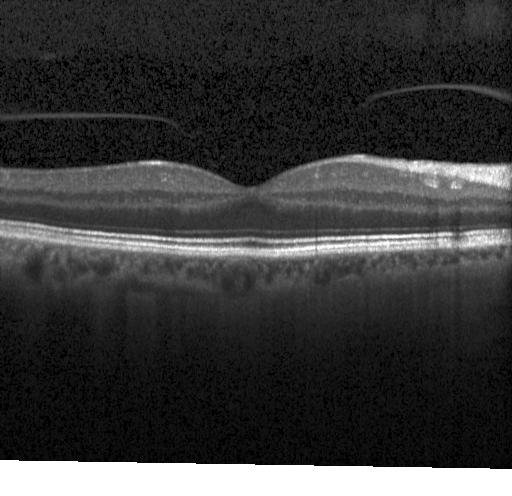

Macular OCT: no choroidal neovascularization, diabetic macular edema, or drusen.